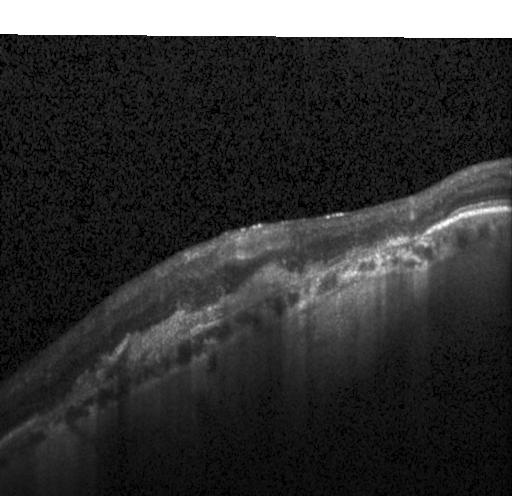 Retinal OCT cross-section; macular scan
Impression: choroidal neovascularization.